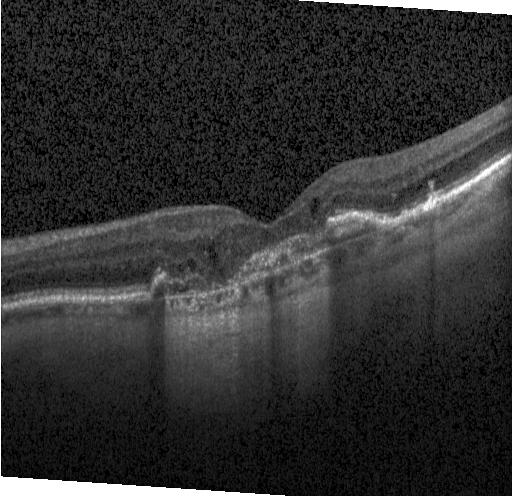

OCT line scan, fovea-centered, SD-OCT. Dx: choroidal neovascularization (CNV).